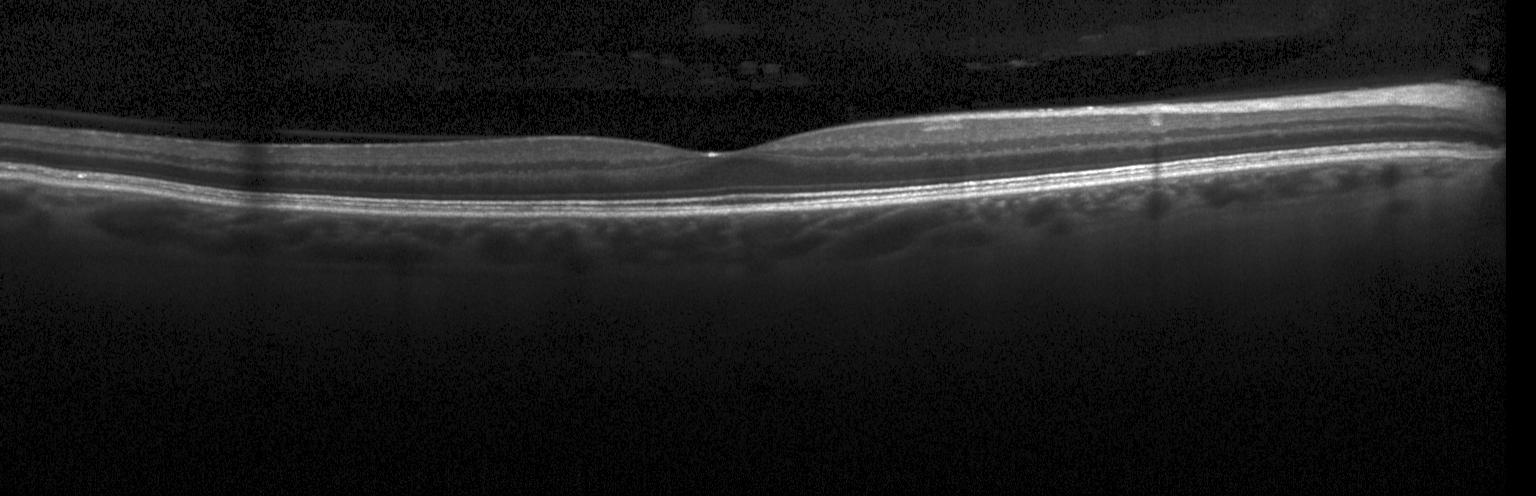

This B-scan demonstrates no CNV, DME, or drusen.